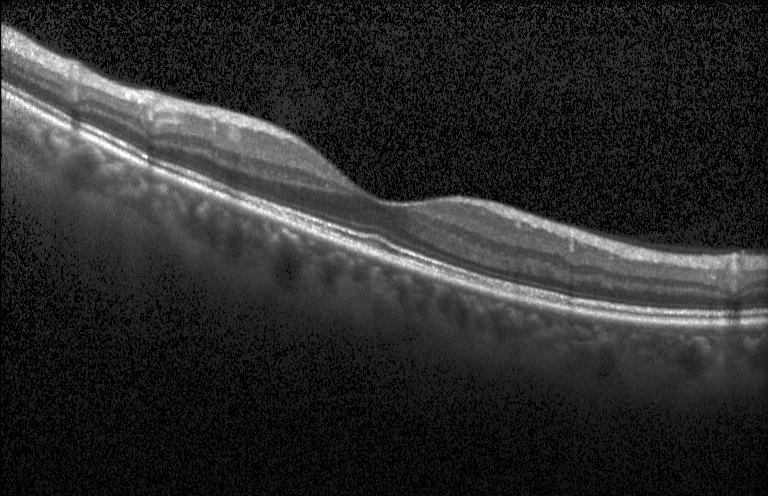
Retinal OCT cross-section, through the macula, spectral-domain OCT, Heidelberg Spectralis. No choroidal neovascularization, no diabetic macular edema, and no drusen.